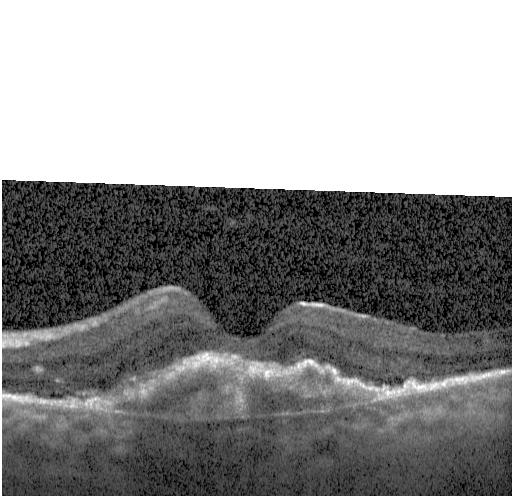
Spectral-domain OCT; Heidelberg Spectralis OCT system; OCT B-scan; horizontal scan through the fovea.
The scan shows a choroidal neovascular membrane.